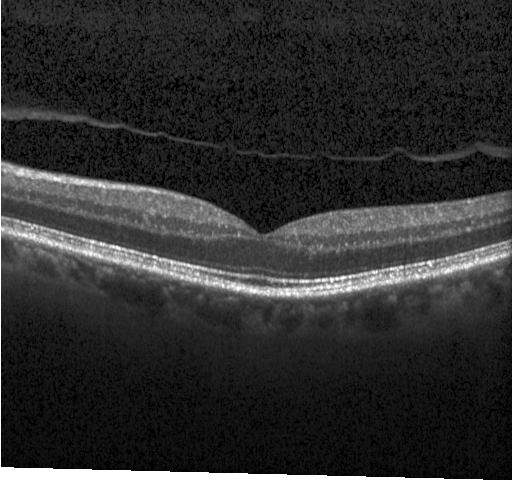

Optical coherence tomography B-scan · spectral-domain OCT. No evidence of CNV, DME, or drusen.